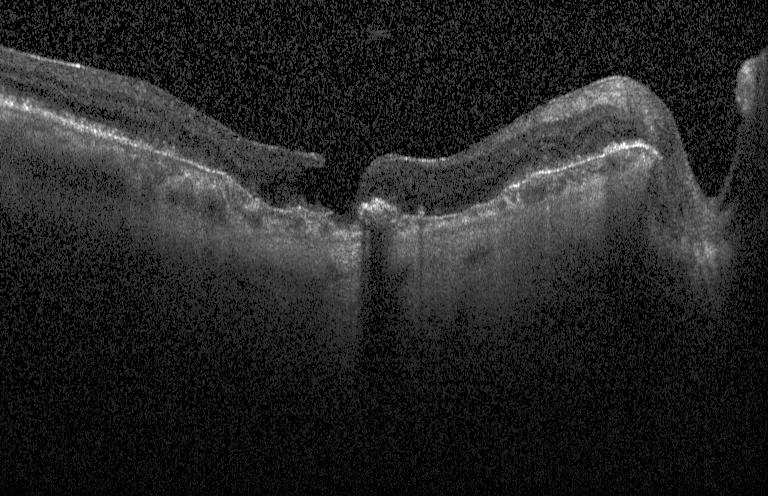

Optical coherence tomography B-scan — This B-scan demonstrates a choroidal neovascular membrane.